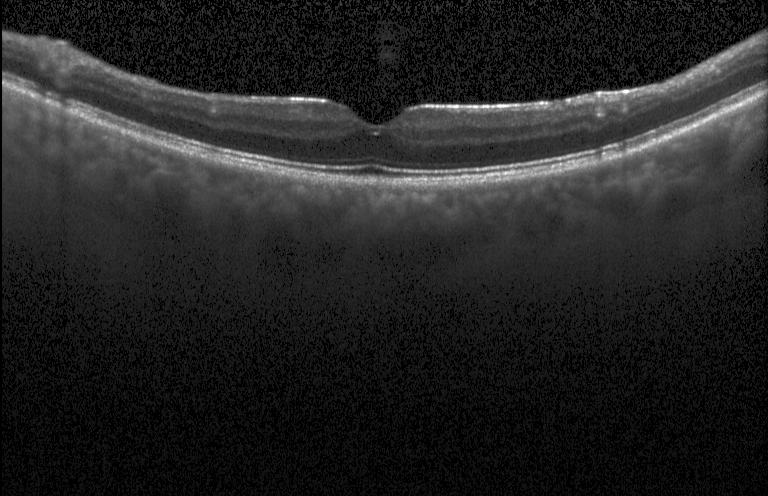
OCT line scan — Impression: no CNV, DME, or drusen.